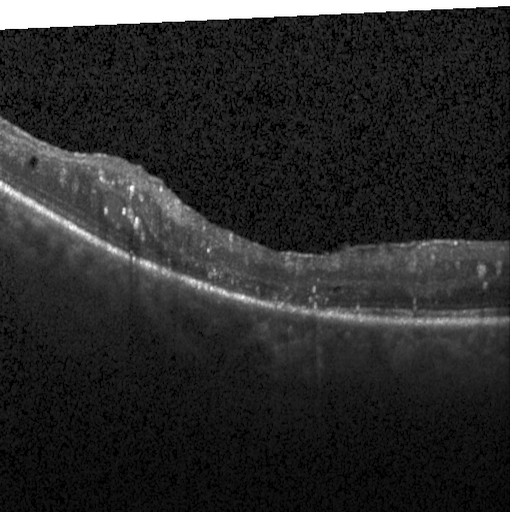
OCT B-scan, Heidelberg Spectralis — Finding: diabetic macular edema.